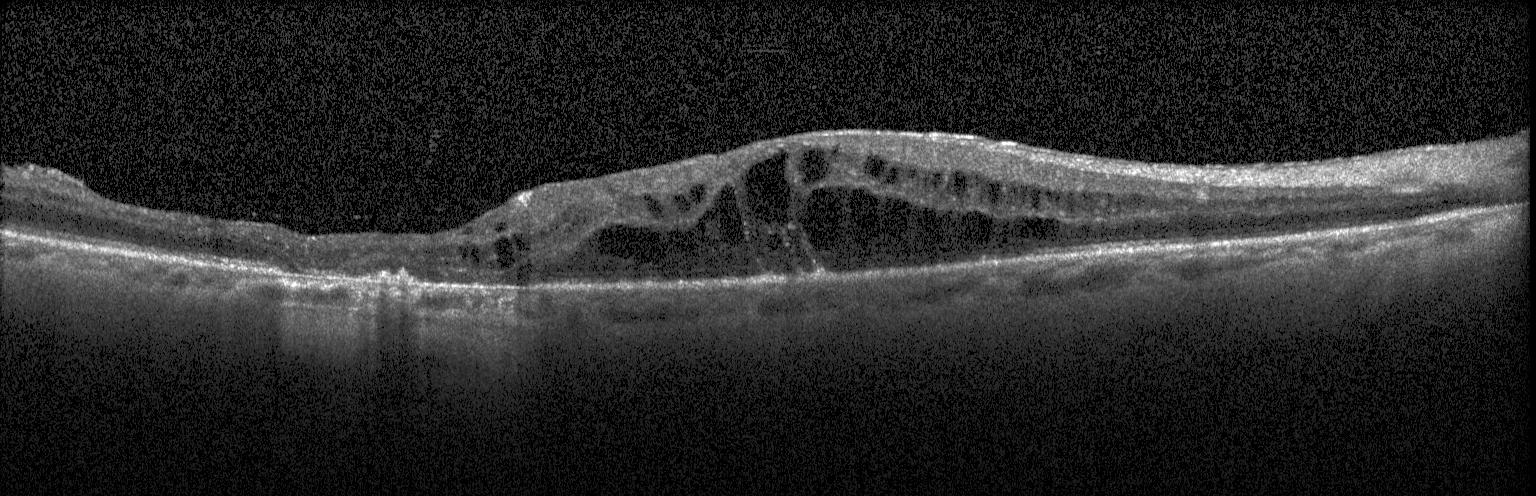
Horizontal scan through the fovea. SD-OCT. Optical coherence tomography B-scan. Diagnosis: diabetic macular edema.